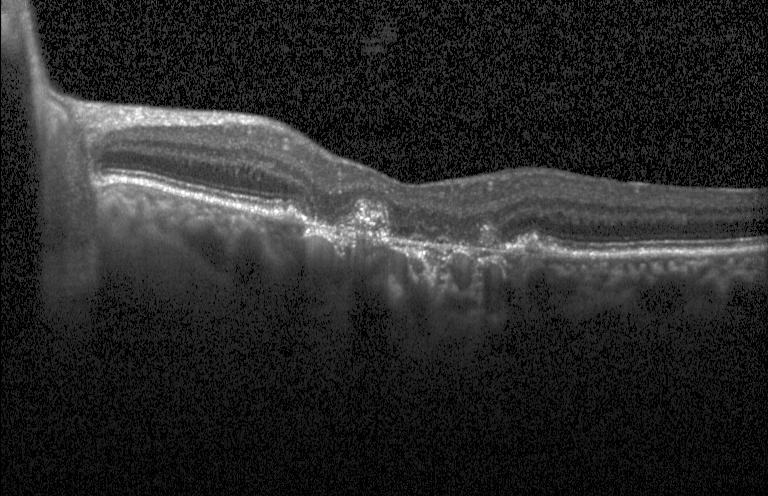
Finding: a choroidal neovascular membrane.